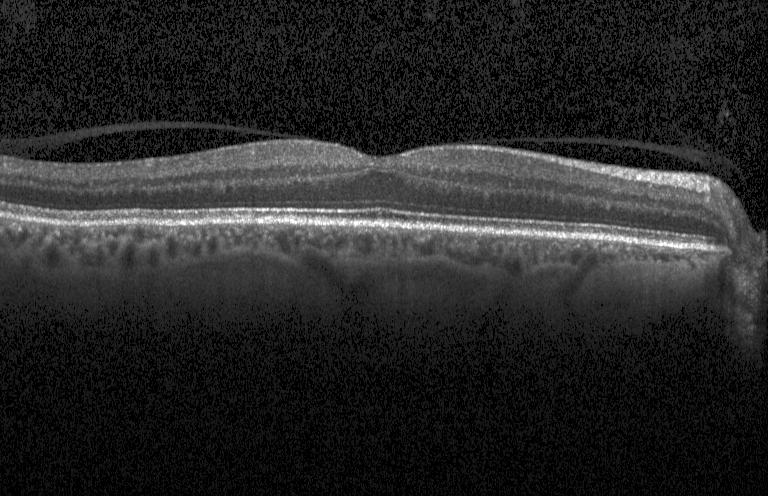
Macular OCT demonstrating no choroidal neovascularization, no diabetic macular edema, and no drusen.